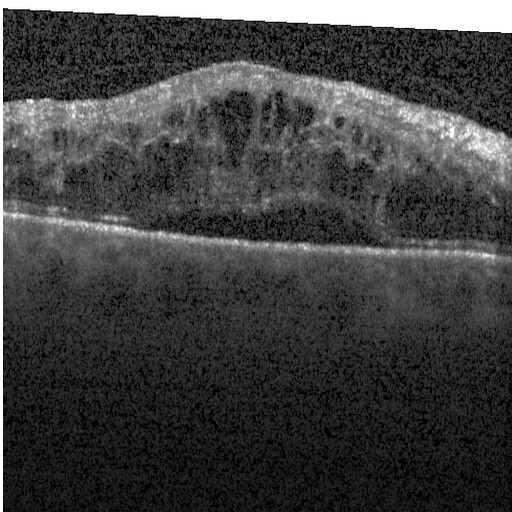

Centered on the fovea; OCT B-scan; spectral-domain OCT; acquired on a Heidelberg Spectralis.
Diagnosis: diabetic macular edema.